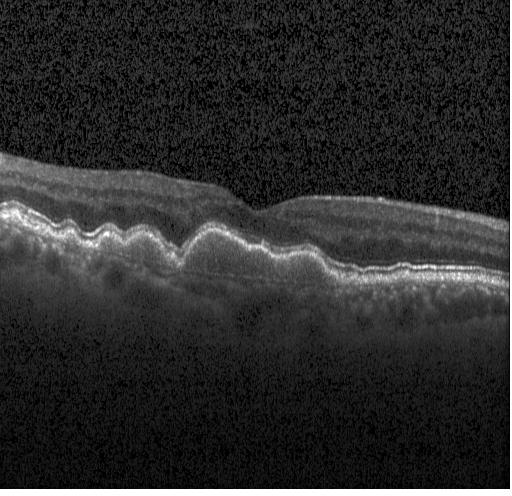 OCT B-scan — Diagnosis: sub-RPE drusenoid deposits.